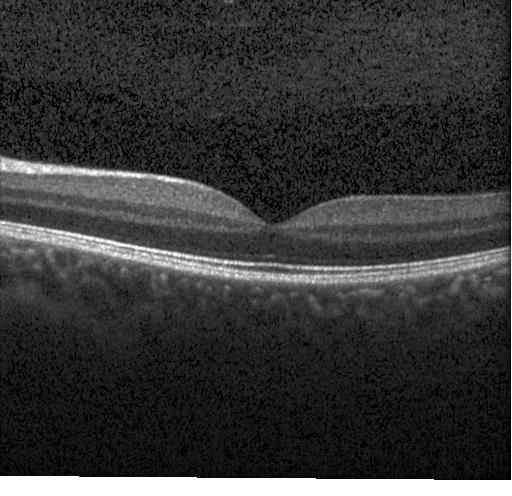 Impression: no evidence of CNV, DME, or drusen.